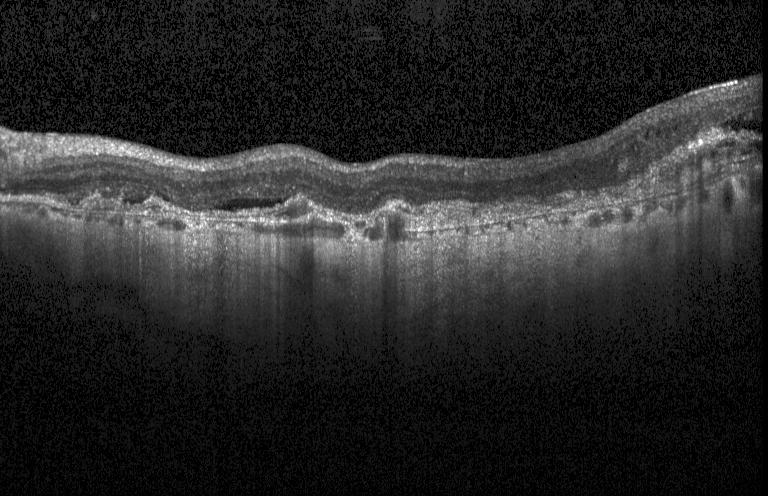 Optical coherence tomography B-scan · Heidelberg Spectralis · through the macula · spectral-domain OCT.
Impression: CNV.